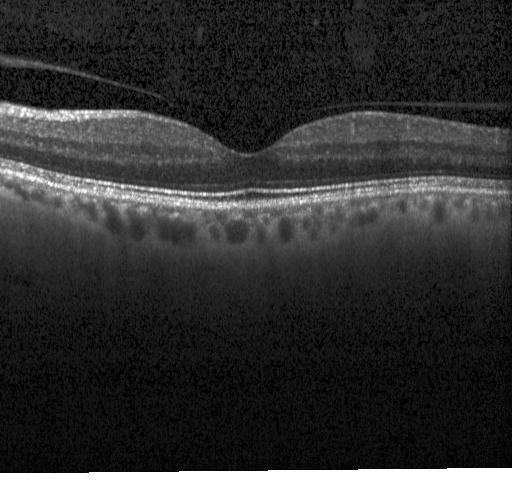

Heidelberg Spectralis, fovea-centered, retinal OCT B-scan.
Finding: no choroidal neovascularization, diabetic macular edema, or drusen.